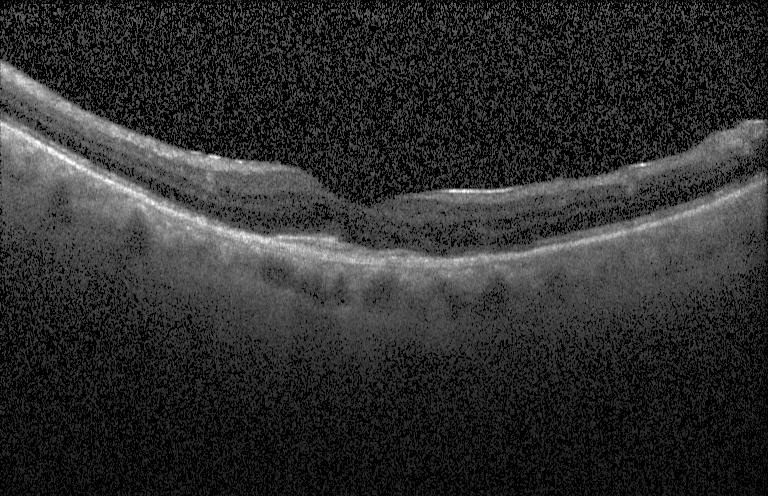 Optical coherence tomography scan
Dx: choroidal neovascularization.